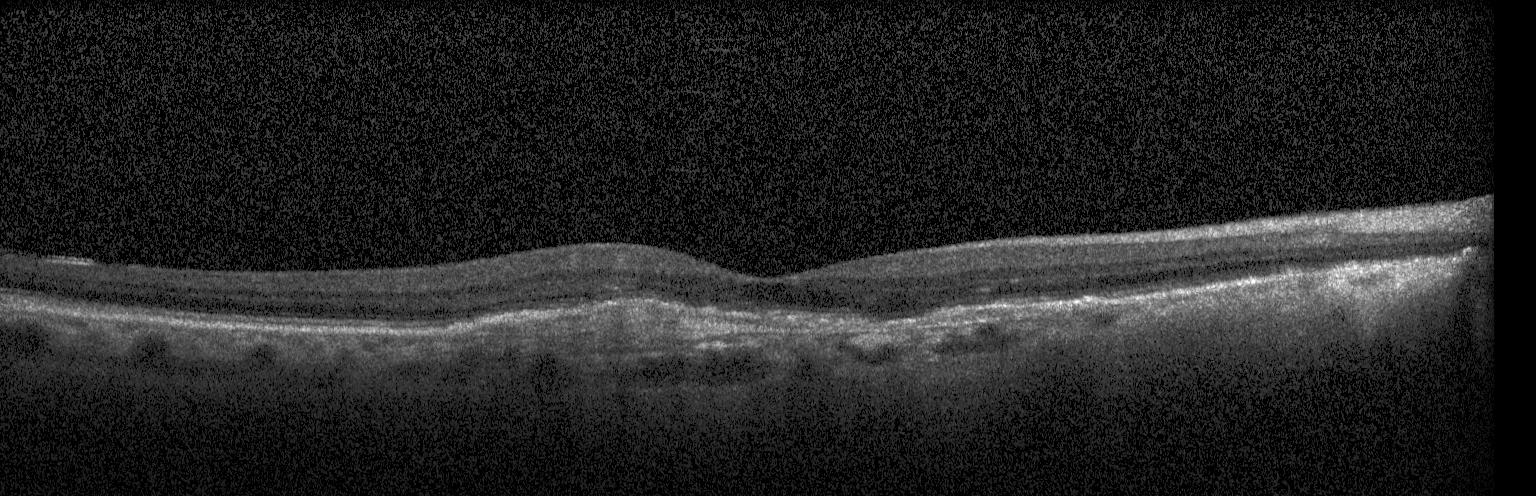 Macular OCT demonstrating a choroidal neovascular membrane.